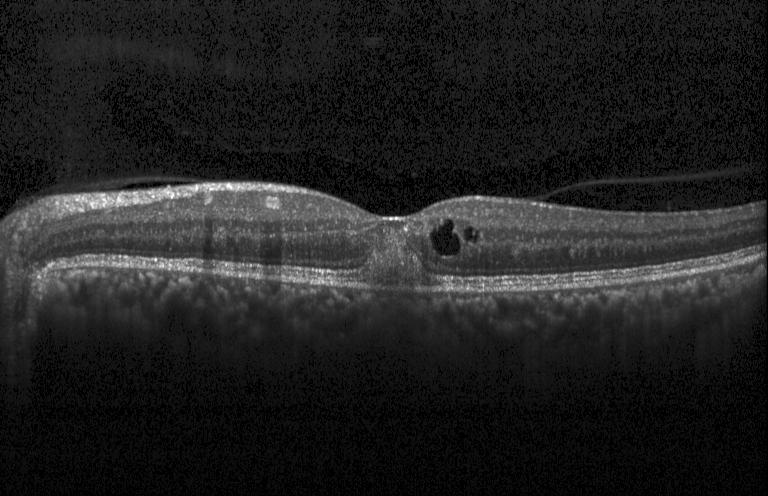
Instrument: Heidelberg Spectralis. Retinal OCT cross-section. SD-OCT — This B-scan demonstrates CNV.